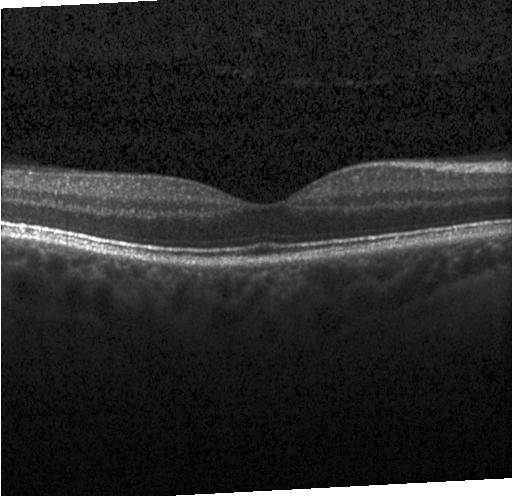
Retinal OCT cross-section showing no choroidal neovascularization, diabetic macular edema, or drusen.